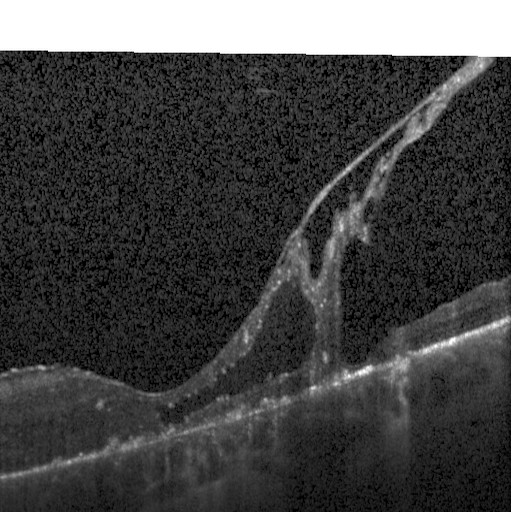 This B-scan demonstrates diabetic macular edema (DME).